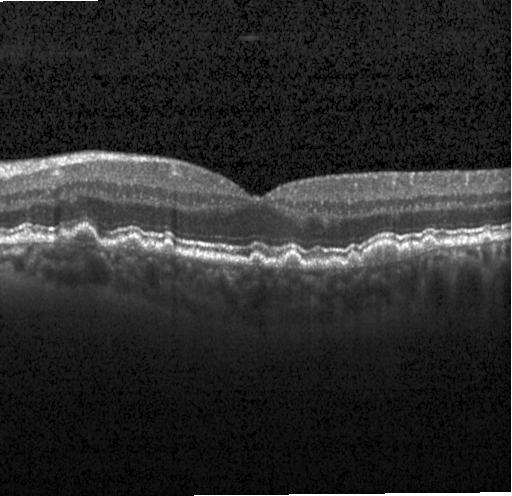

Retinal OCT cross-section — Assessment: sub-RPE drusenoid deposits.